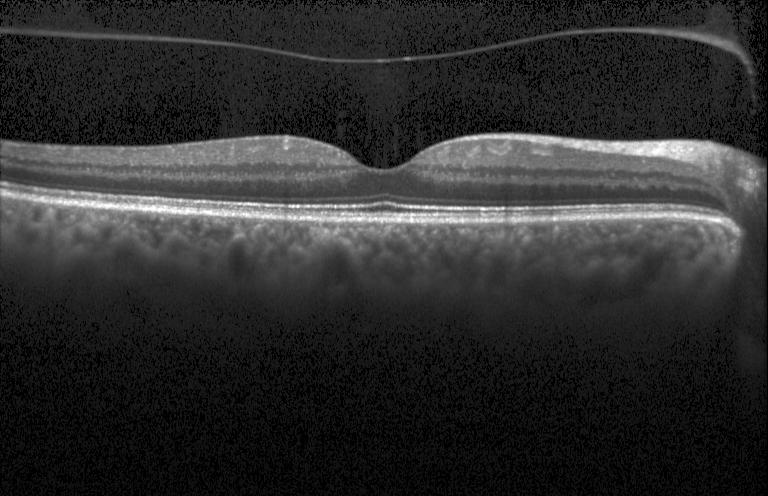

SD-OCT; OCT line scan; through the macula.
This B-scan demonstrates no evidence of choroidal neovascularization, diabetic macular edema, or drusen.